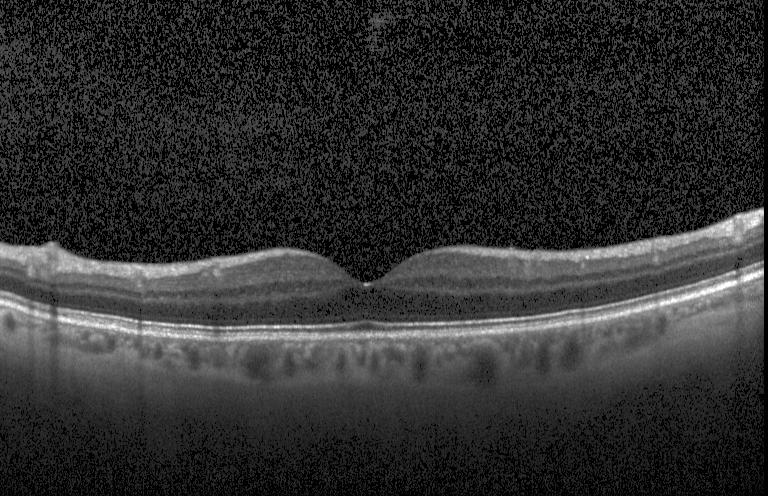 SD-OCT, macular scan, OCT line scan, Heidelberg Spectralis OCT system
Neither choroidal neovascularization, diabetic macular edema, nor drusen.